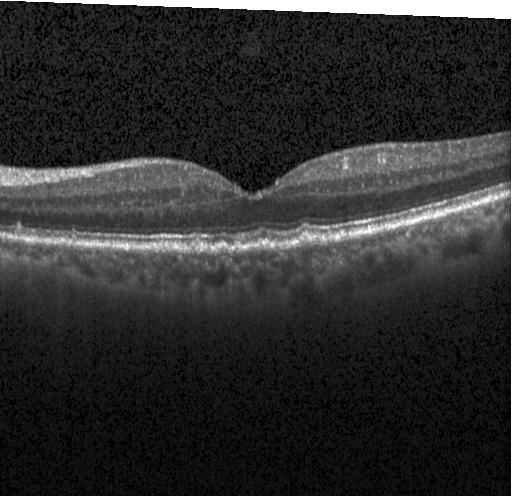
Optical coherence tomography scan
Diagnosis: sub-RPE drusenoid deposits.